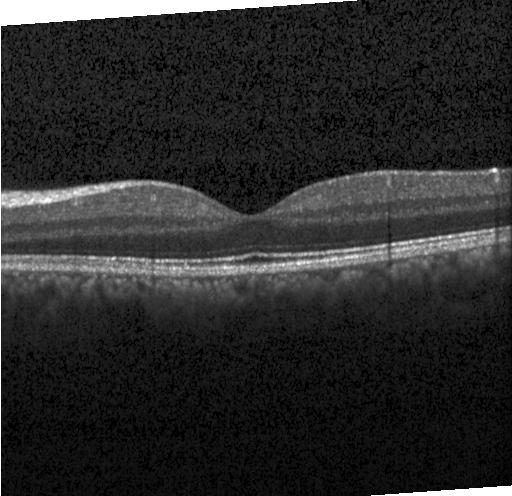

Finding: no choroidal neovascularization, no diabetic macular edema, and no drusen.